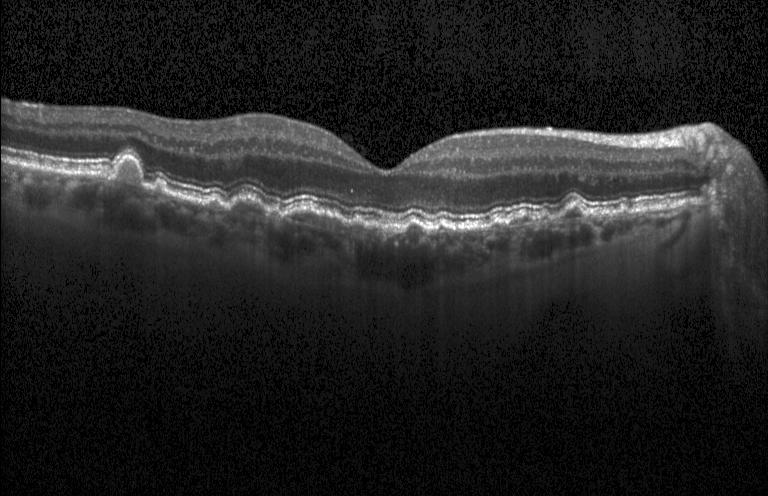

OCT line scan. Heidelberg Spectralis. Centered on the fovea. Spectral-domain optical coherence tomography — Impression: sub-RPE drusenoid deposits.